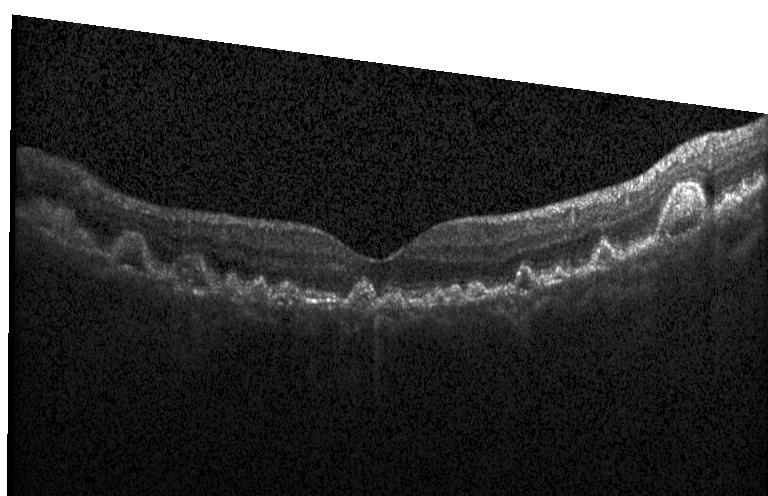 The scan shows a choroidal neovascular membrane.